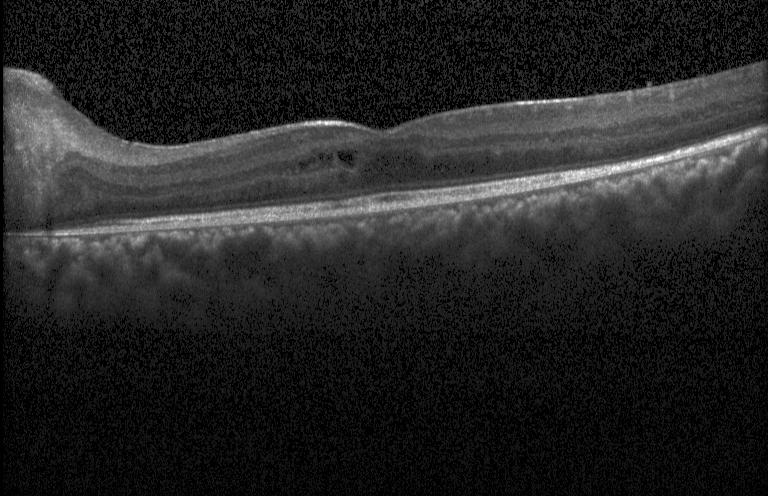
Diagnosis: DME.